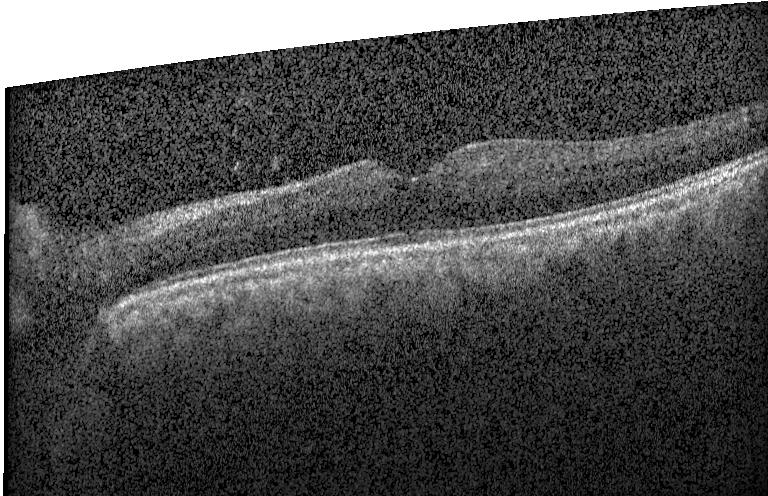

Assessment: no evidence of choroidal neovascularization, diabetic macular edema, or drusen.